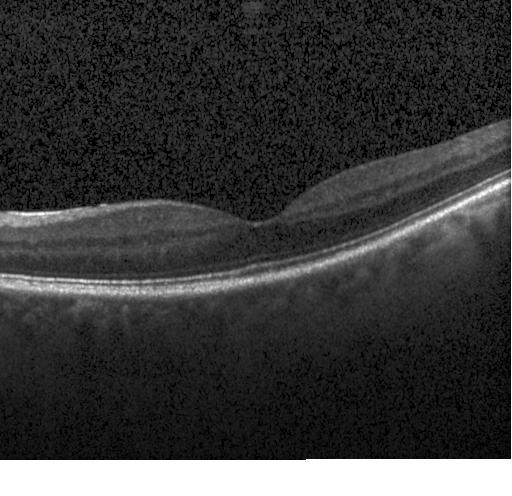 Retinal OCT B-scan, horizontal scan through the fovea, Heidelberg Spectralis OCT system. Impression: neither CNV, DME, nor drusen.